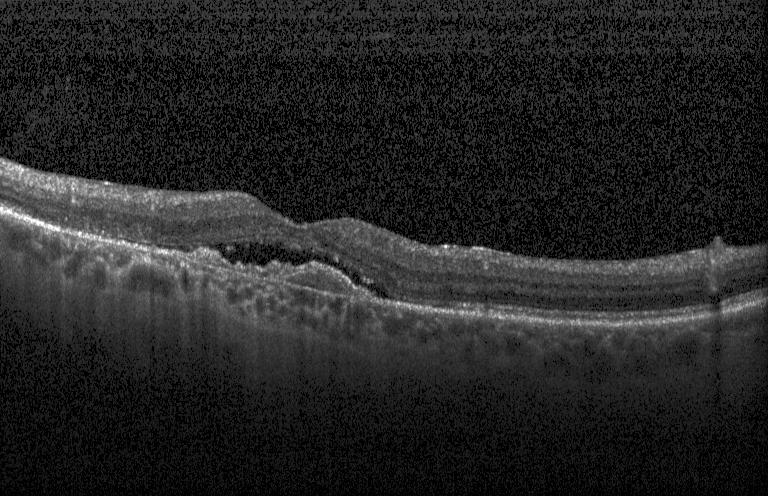
Through the macula; spectral-domain optical coherence tomography; retinal OCT B-scan; instrument: Heidelberg Spectralis — Dx: choroidal neovascularization (CNV).